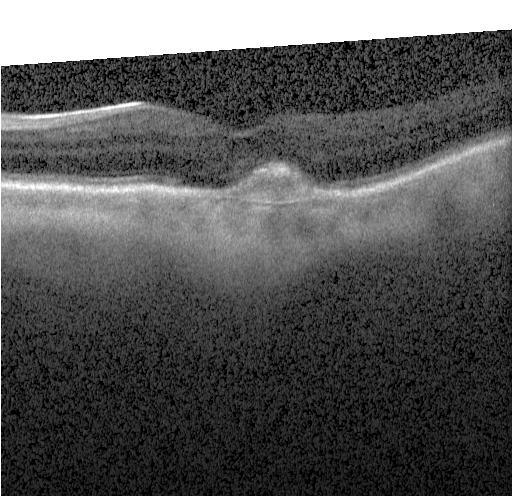

Instrument: Heidelberg Spectralis. Fovea-centered. OCT line scan
Impression: CNV.